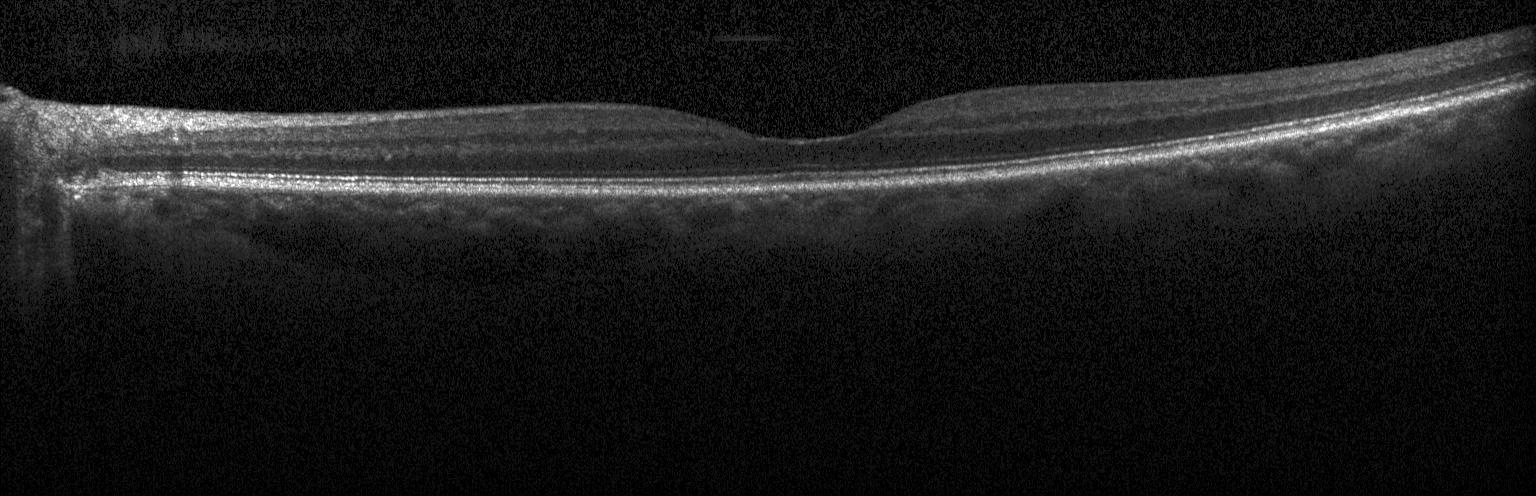
Diagnosis: neither choroidal neovascularization, diabetic macular edema, nor drusen.